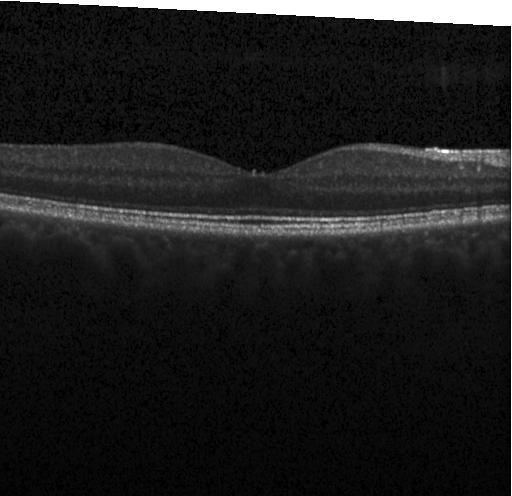
OCT B-scan · spectral-domain OCT · through the macula
Impression: no choroidal neovascularization, no diabetic macular edema, and no drusen.